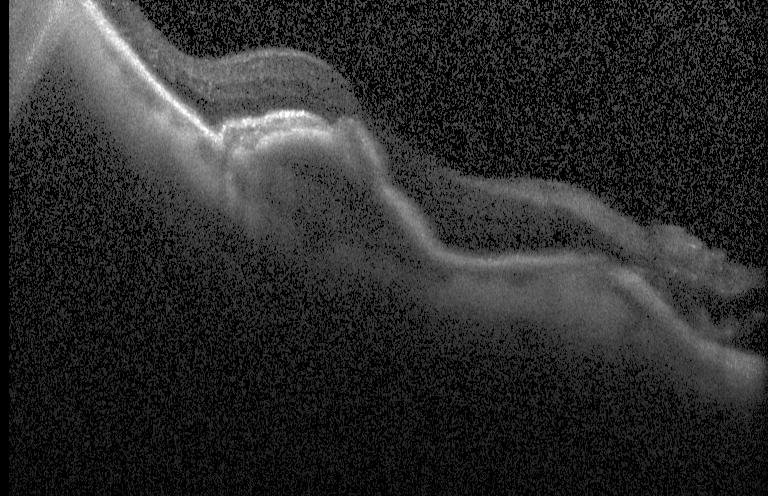
Retinal OCT cross-section. Fovea-centered. Spectral-domain optical coherence tomography.
A choroidal neovascular membrane.